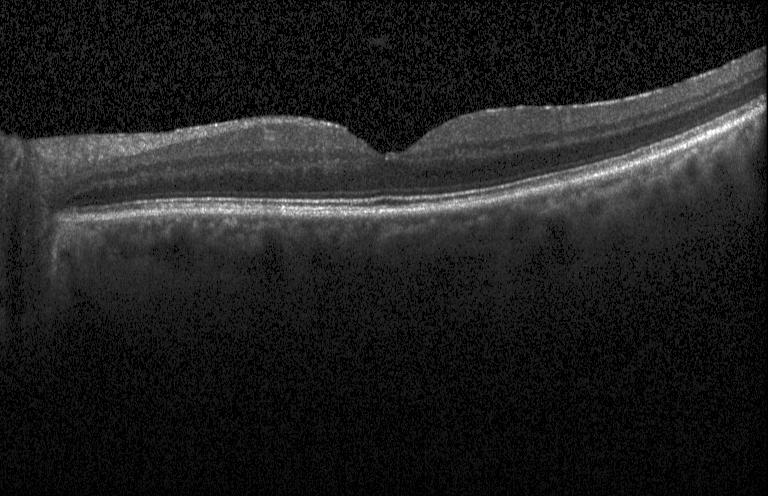
Retinal OCT cross-section.
Assessment: neither choroidal neovascularization, diabetic macular edema, nor drusen.